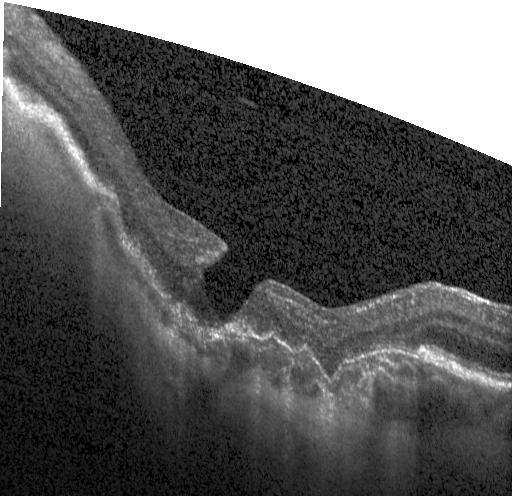 OCT line scan, Heidelberg Spectralis OCT system — Dx: a choroidal neovascular membrane.